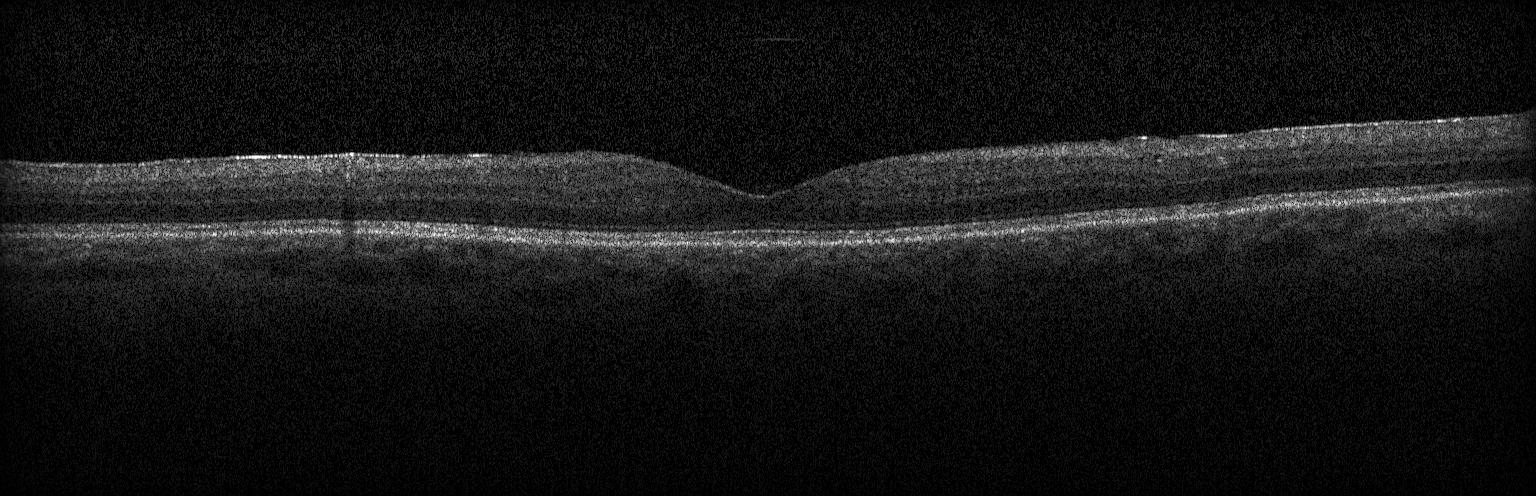

Neither choroidal neovascularization, diabetic macular edema, nor drusen.